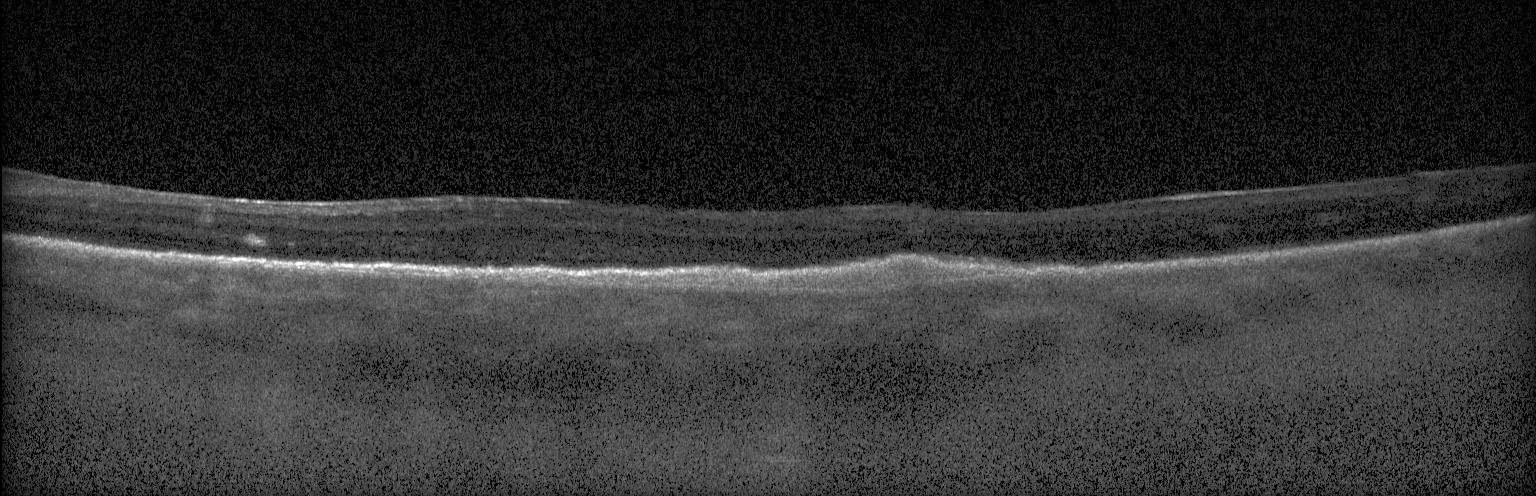
Retinal OCT cross-section, spectral-domain optical coherence tomography, through the macula.
Diagnosis: a choroidal neovascular membrane.